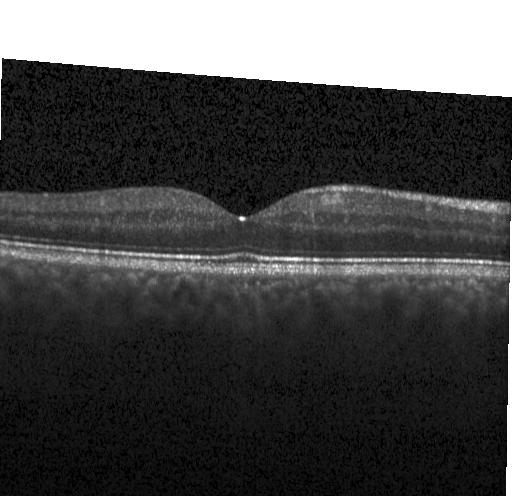

Spectral-domain OCT · retinal OCT B-scan · centered on the fovea
Neither choroidal neovascularization, diabetic macular edema, nor drusen.